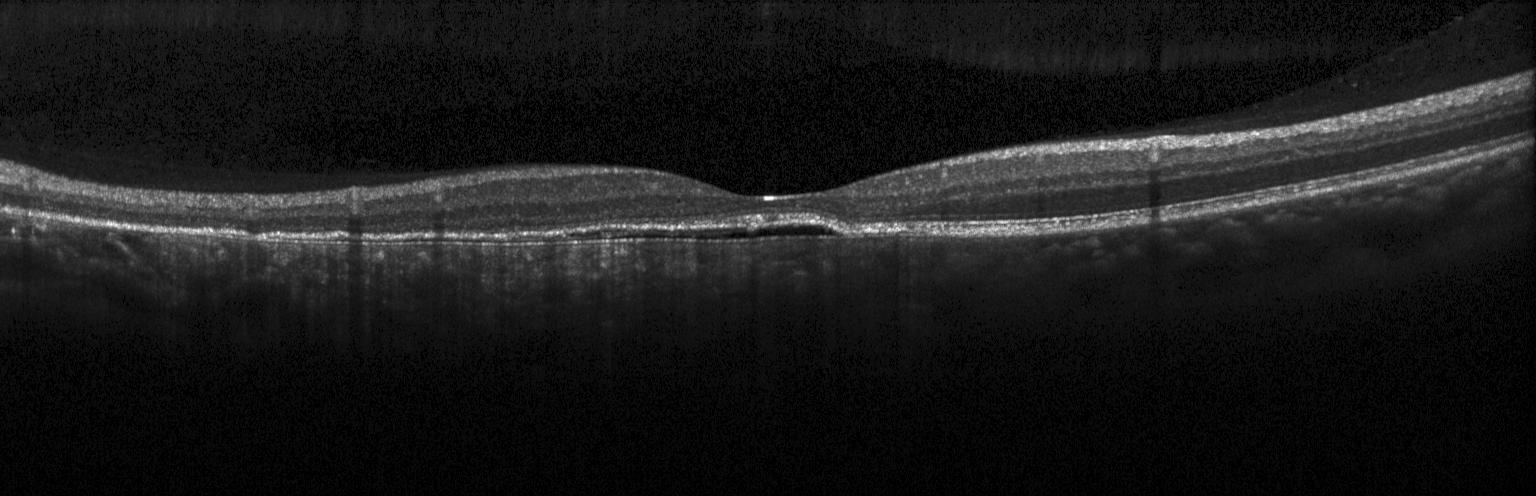 OCT line scan — Assessment: choroidal neovascularization.